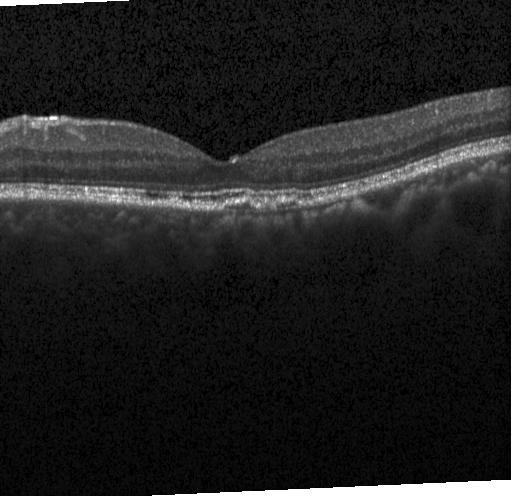 Retinal OCT B-scan
Finding: sub-RPE drusenoid deposits.